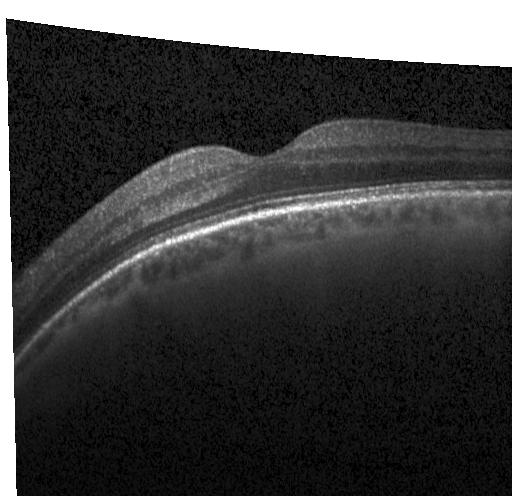 Macular scan · acquired on a Heidelberg Spectralis · OCT line scan · spectral-domain OCT
Dx: no CNV, no DME, and no drusen.